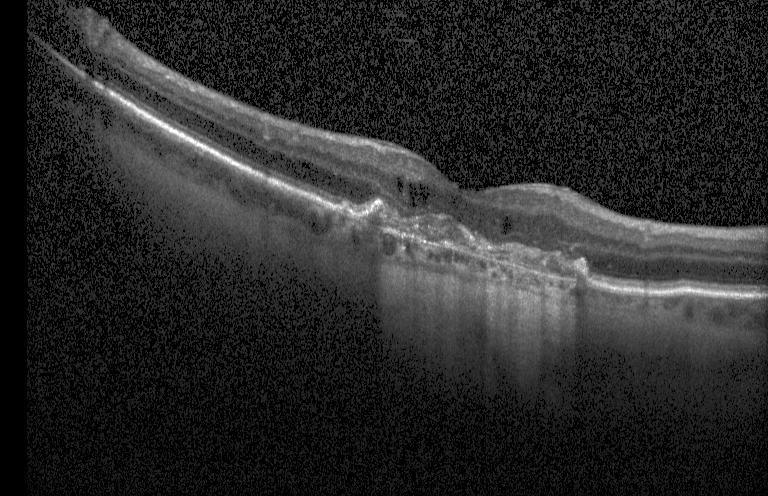
Impression: a choroidal neovascular membrane.